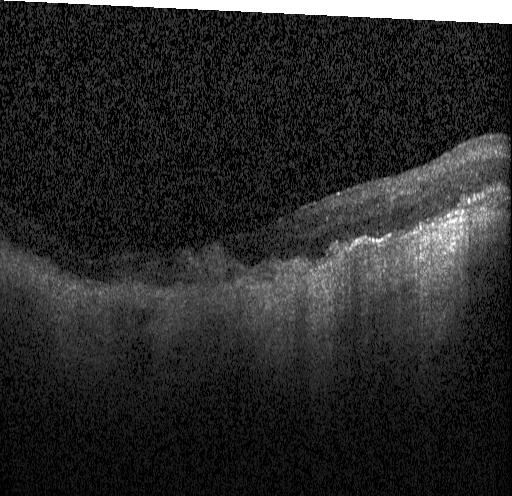 Optical coherence tomography B-scan
Impression: choroidal neovascularization (CNV).